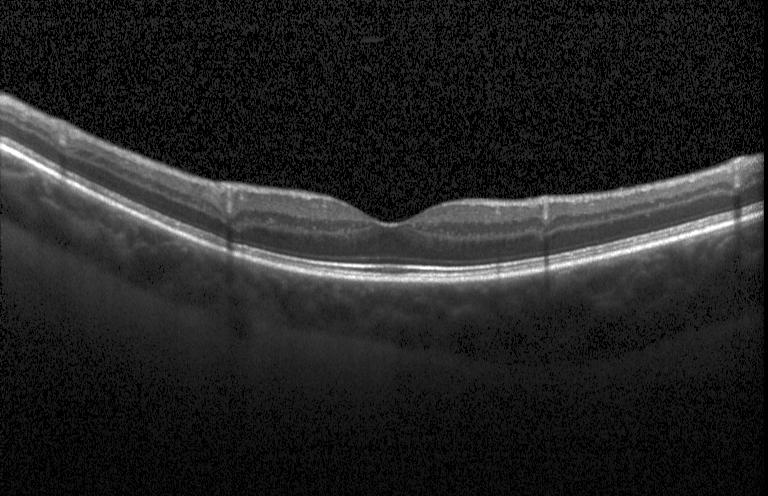
Centered on the fovea. Retinal OCT B-scan.
Diagnosis: no choroidal neovascularization, no diabetic macular edema, and no drusen.